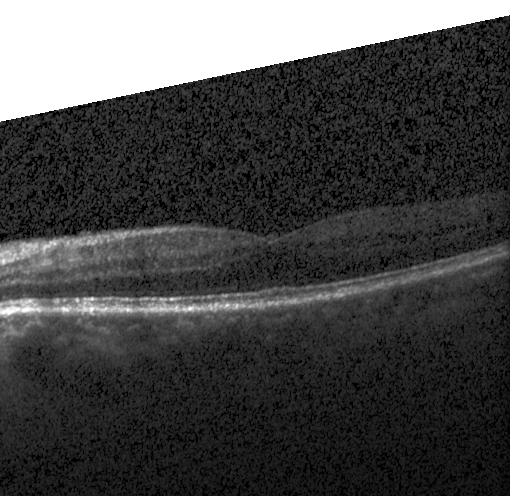 Centered on the fovea; retinal OCT cross-section; acquired on a Heidelberg Spectralis. Finding: no choroidal neovascularization, no diabetic macular edema, and no drusen.